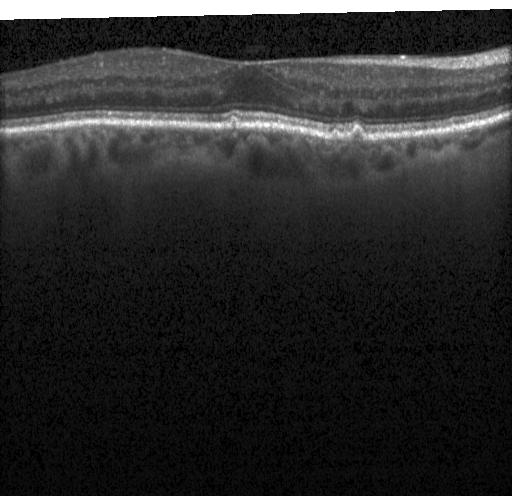

Dx: multiple drusen.